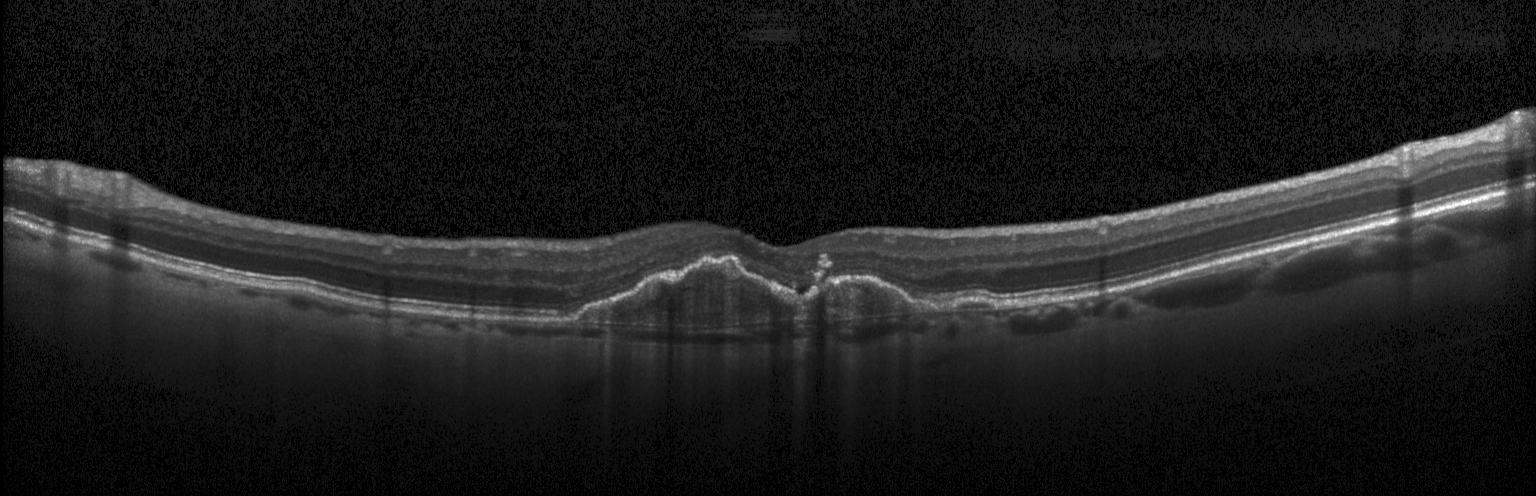 The scan shows choroidal neovascularization (CNV).